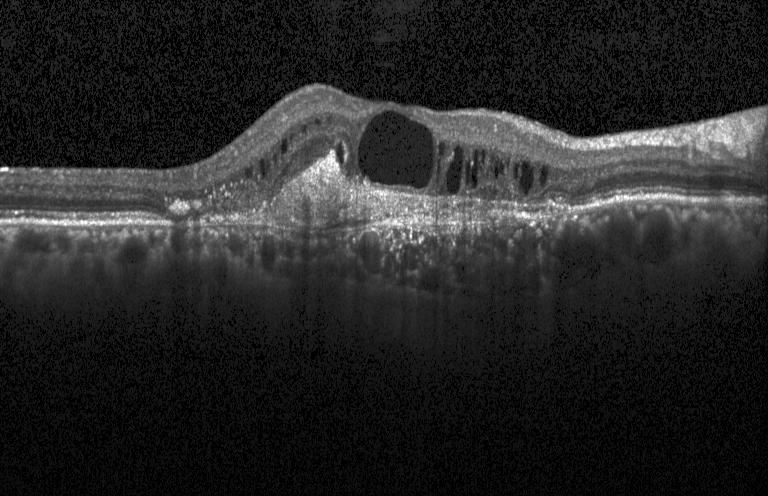 Macular OCT: CNV.